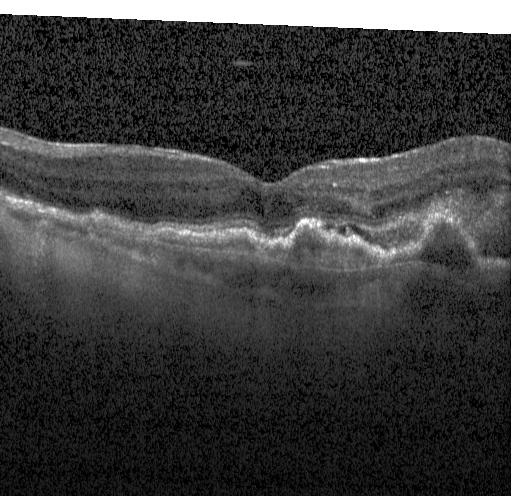
Optical coherence tomography scan — Impression: choroidal neovascularization.